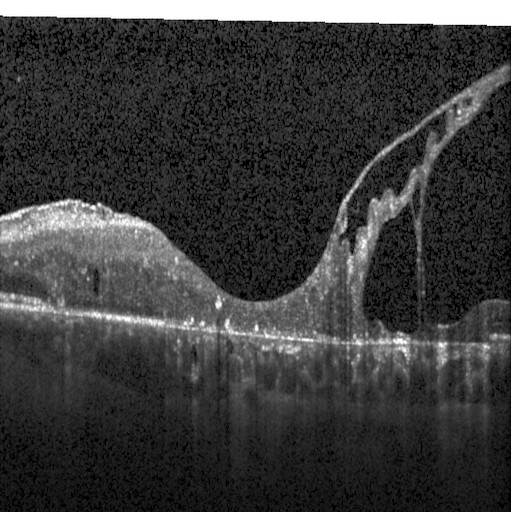 Heidelberg Spectralis · OCT line scan.
Diabetic macular edema.